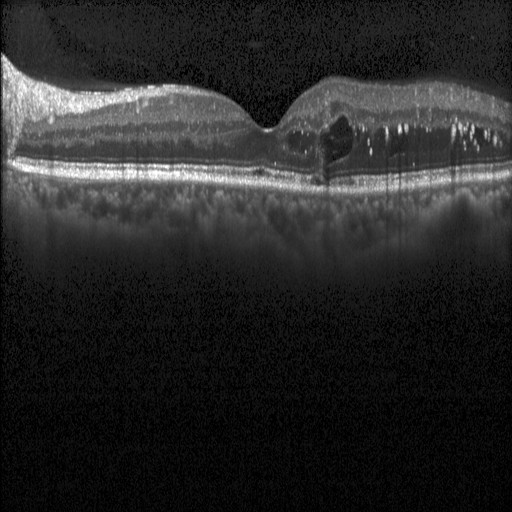
OCT finding: diabetic macular edema.